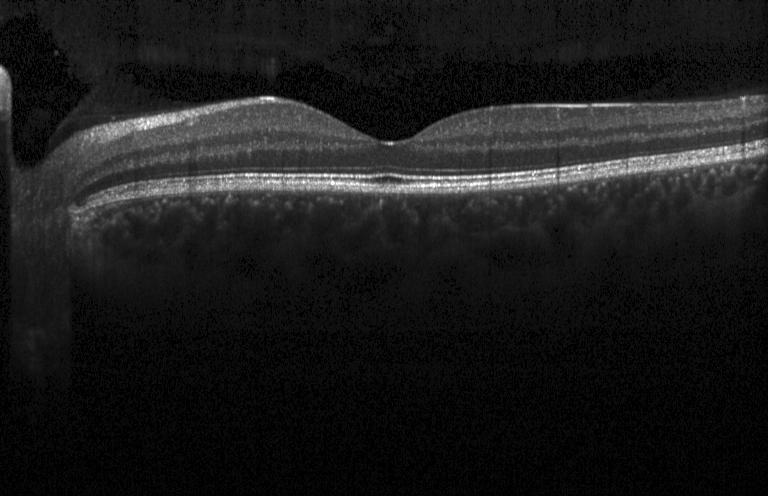
OCT B-scan, fovea-centered
Finding: no choroidal neovascularization, no diabetic macular edema, and no drusen.